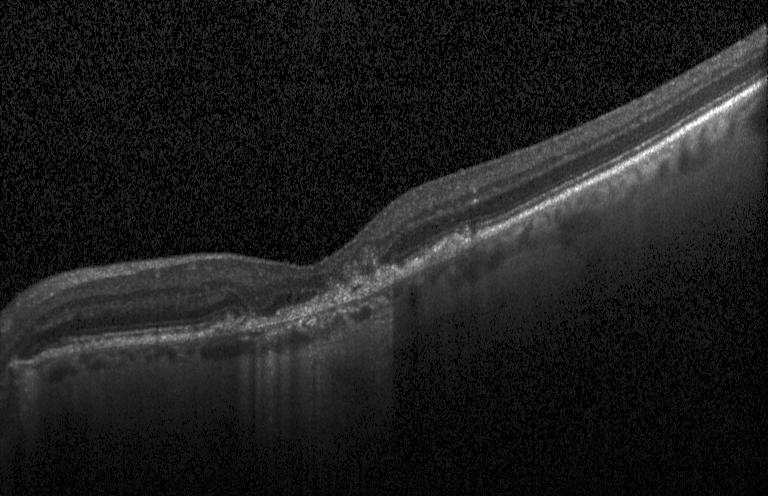 OCT B-scan · centered on the fovea.
Diagnosis: a choroidal neovascular membrane.